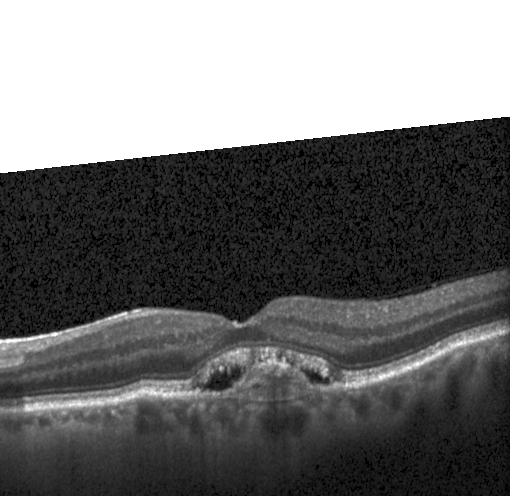 Diagnosis: a choroidal neovascular membrane.